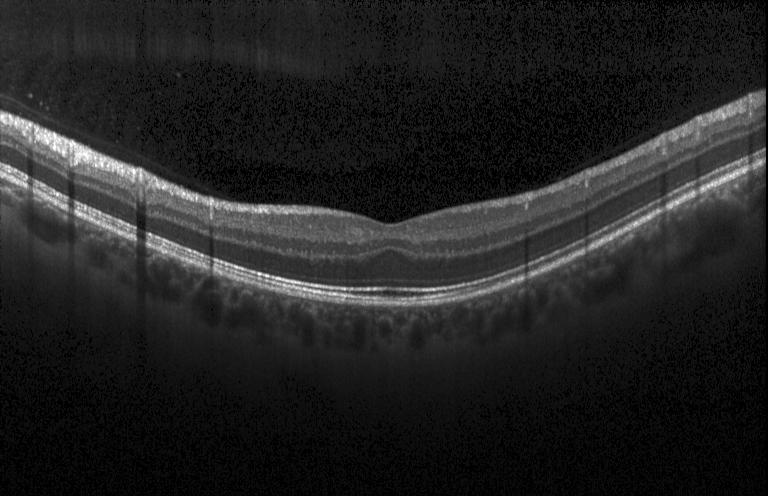

Assessment: neither CNV, DME, nor drusen.